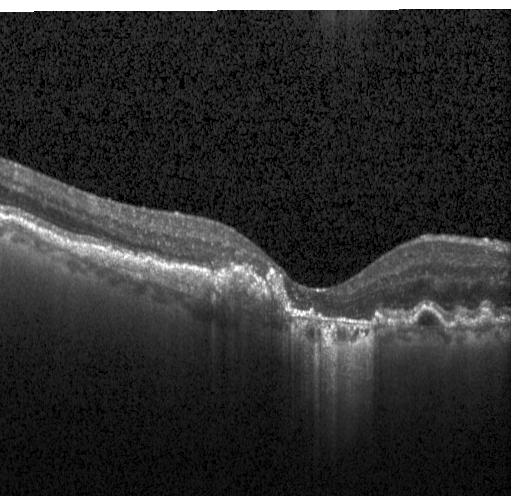

Optical coherence tomography B-scan · centered on the fovea. Dx: a choroidal neovascular membrane.